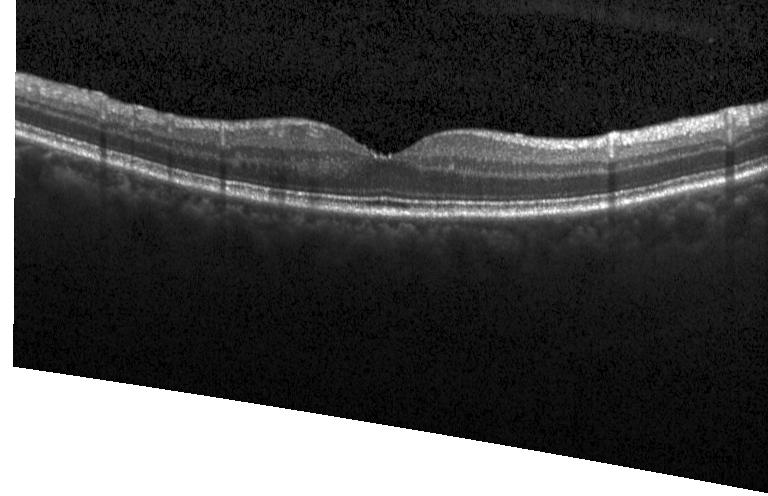
Retinal OCT B-scan
Dx: neither choroidal neovascularization, diabetic macular edema, nor drusen.